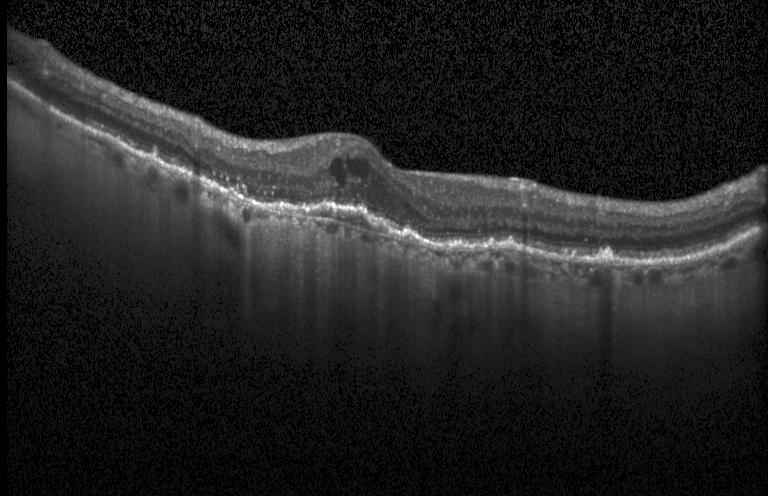

Heidelberg Spectralis OCT system, macular scan, optical coherence tomography B-scan.
Assessment: a choroidal neovascular membrane.